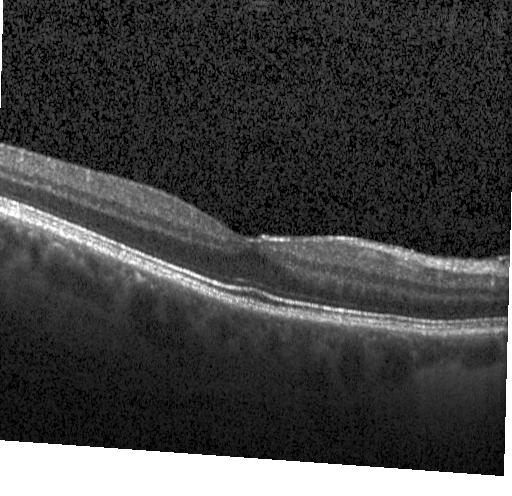 OCT scan showing no evidence of CNV, DME, or drusen.